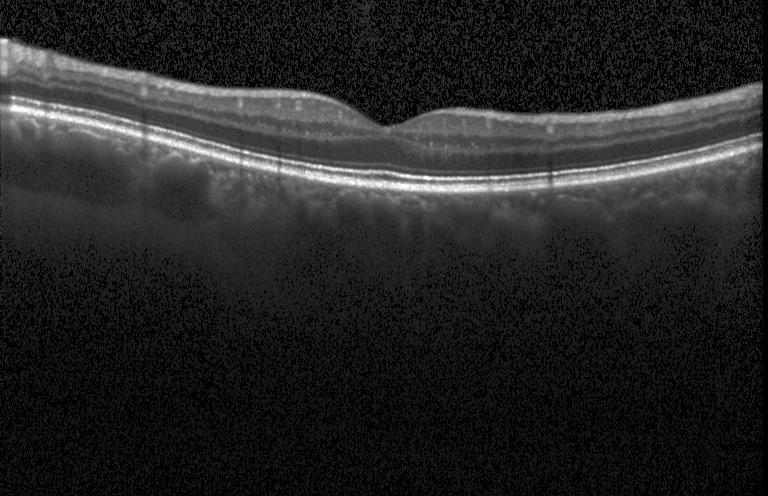

Fovea-centered, optical coherence tomography B-scan. OCT finding: neither choroidal neovascularization, diabetic macular edema, nor drusen.